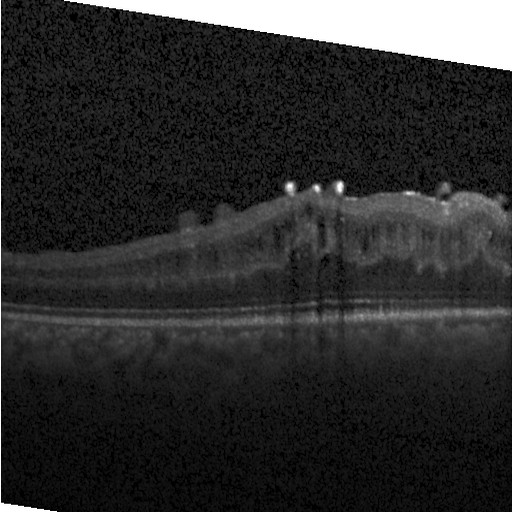 Heidelberg Spectralis; retinal OCT B-scan — Diagnosis: diabetic macular edema (DME).